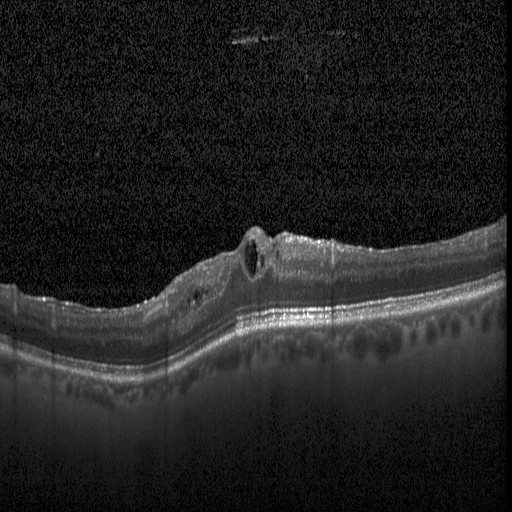 Macular OCT demonstrating DME.